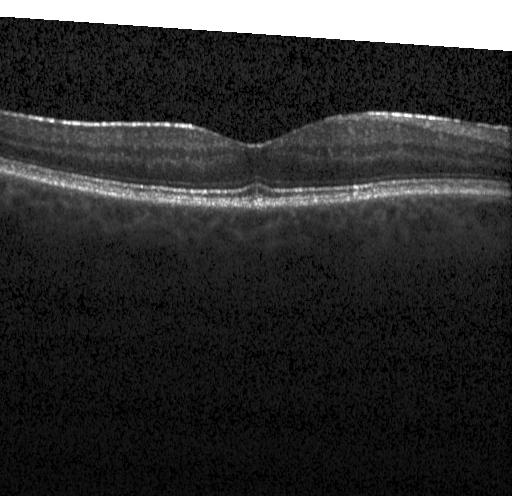
Macular OCT: no choroidal neovascularization, no diabetic macular edema, and no drusen.